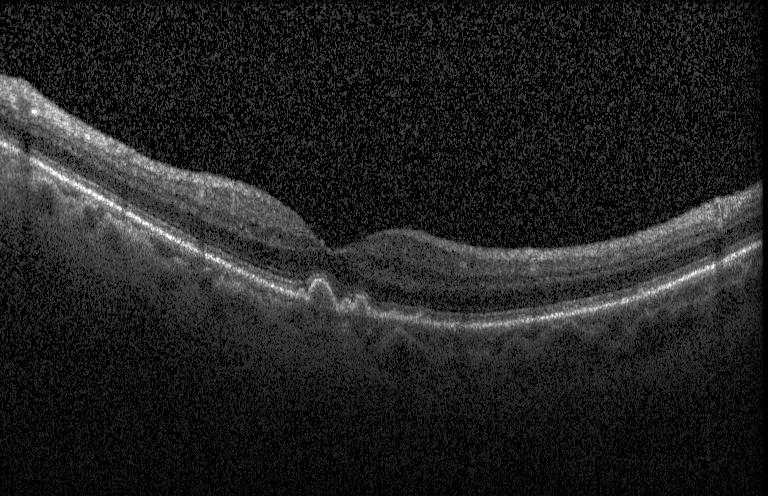 OCT B-scan showing sub-RPE drusenoid deposits.